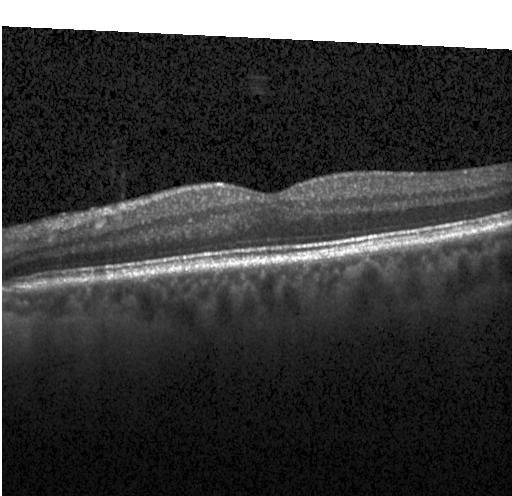 Centered on the fovea. OCT B-scan. SD-OCT — Assessment: neither choroidal neovascularization, diabetic macular edema, nor drusen.